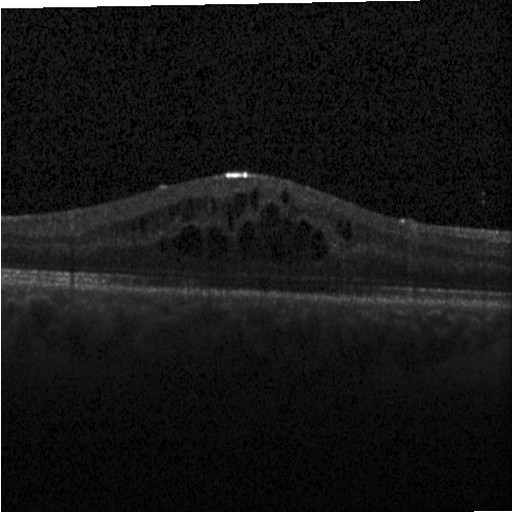
Instrument: Heidelberg Spectralis, through the macula, OCT line scan, spectral-domain optical coherence tomography — Diabetic macular edema.